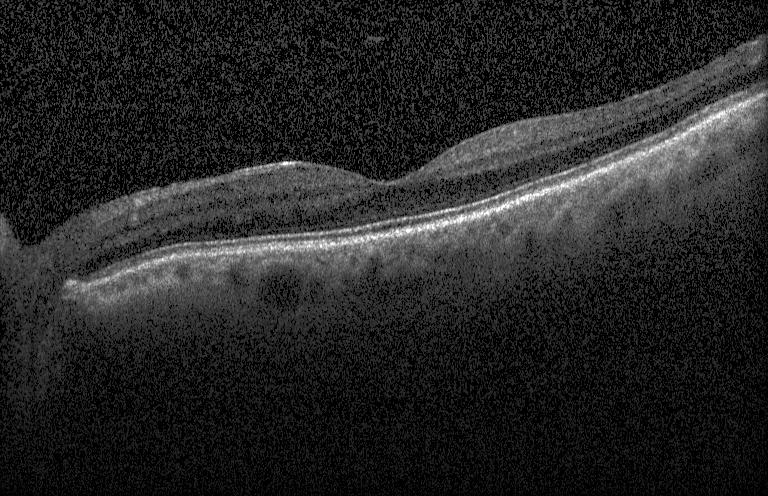 Centered on the fovea · retinal OCT B-scan · spectral-domain OCT. Finding: no choroidal neovascularization, no diabetic macular edema, and no drusen.